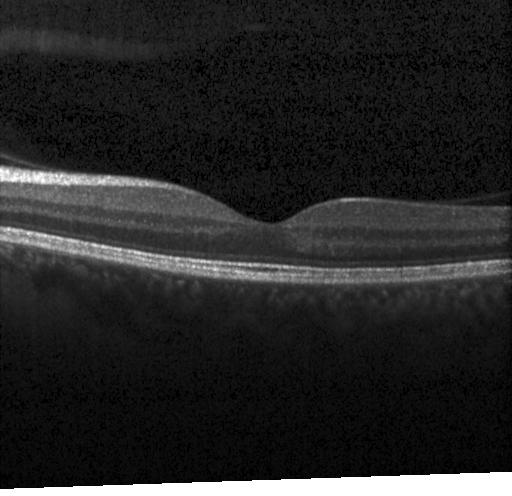

Retinal OCT cross-section; centered on the fovea; spectral-domain optical coherence tomography.
Macular OCT: neither choroidal neovascularization, diabetic macular edema, nor drusen.